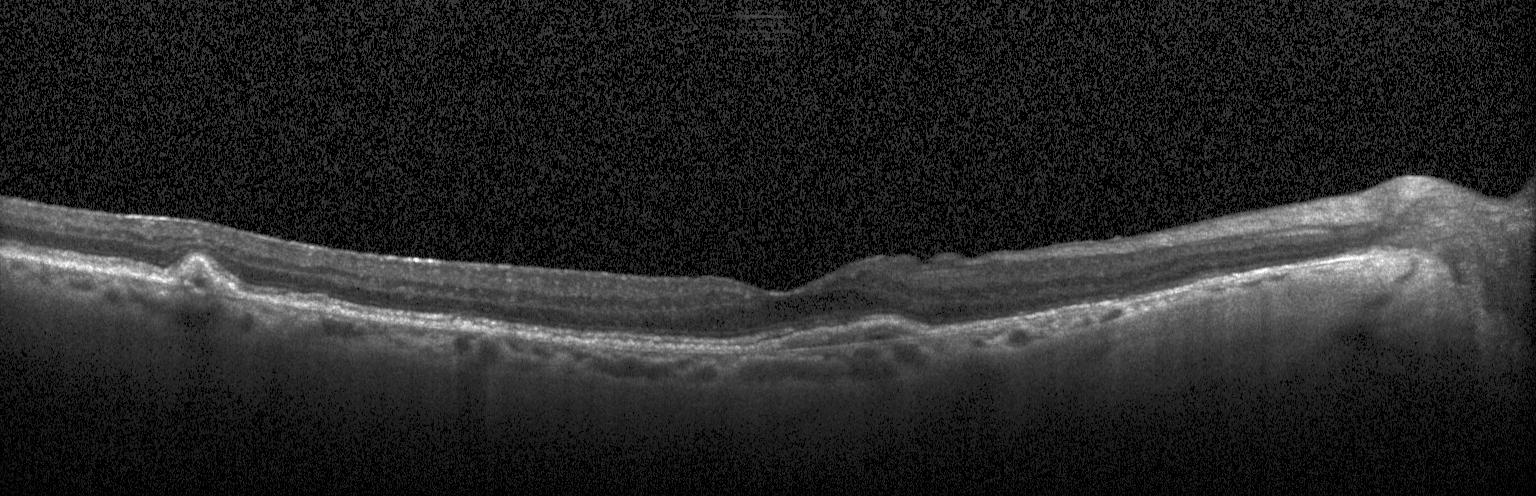
Optical coherence tomography B-scan.
Assessment: a choroidal neovascular membrane.